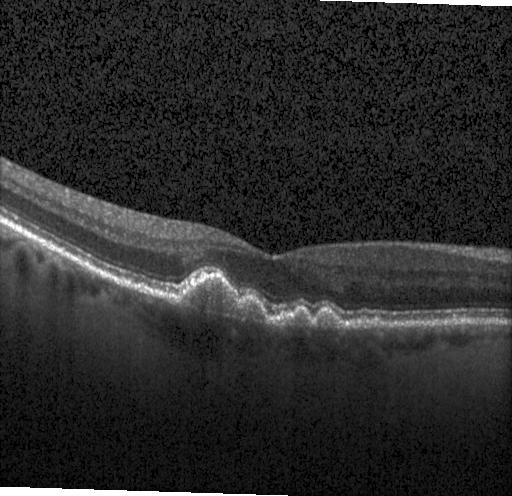
Diagnosis: multiple drusen.